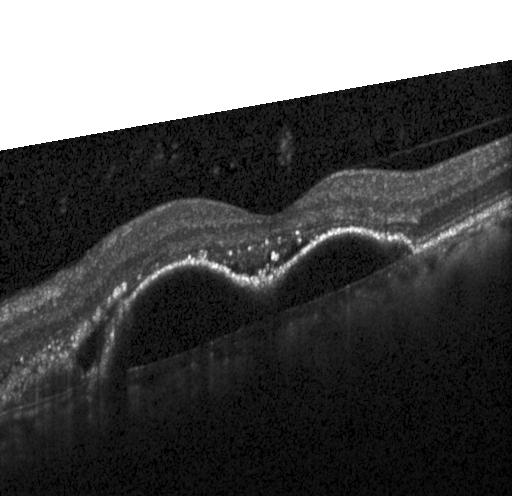 A choroidal neovascular membrane.